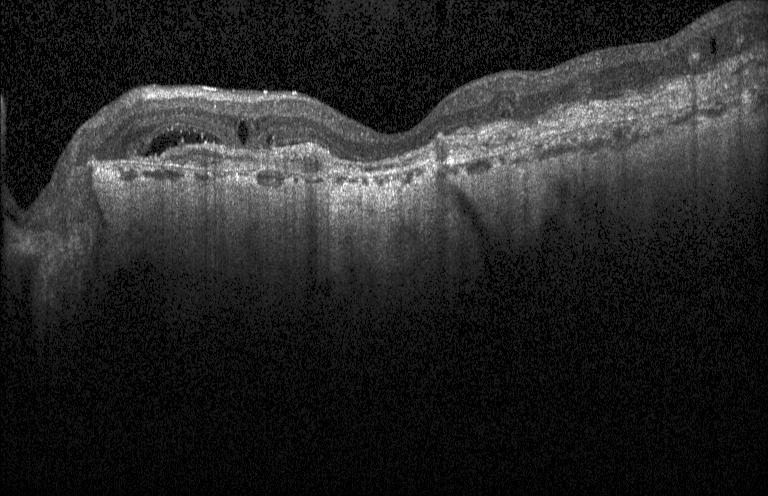

Impression: a choroidal neovascular membrane.